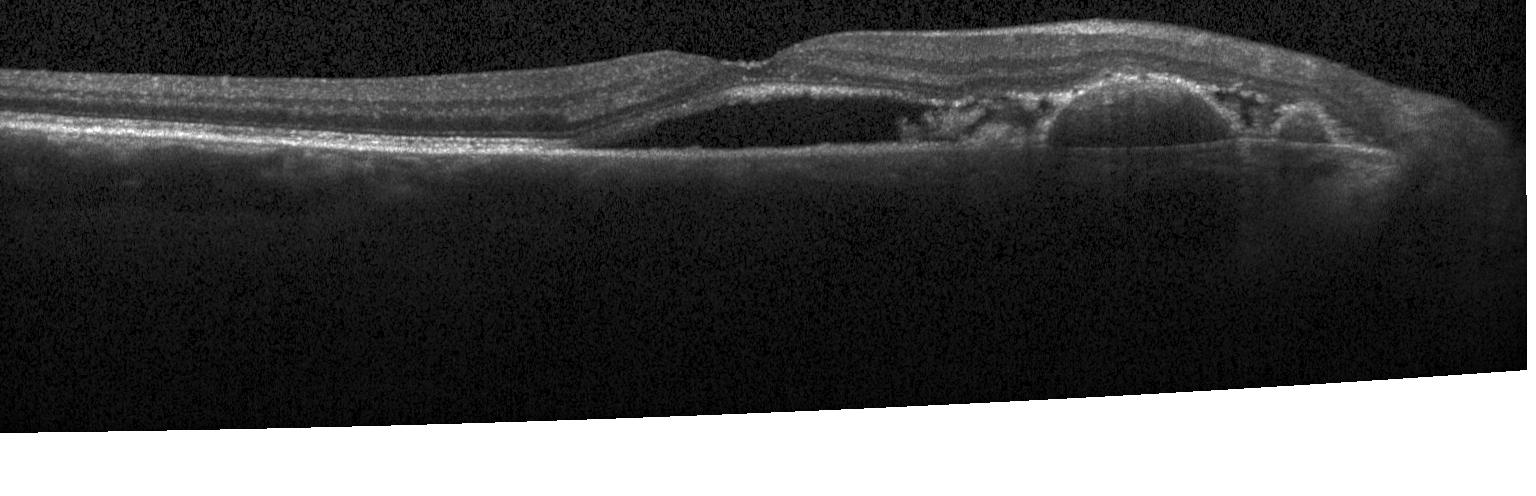
Retinal OCT cross-section showing choroidal neovascularization (CNV).